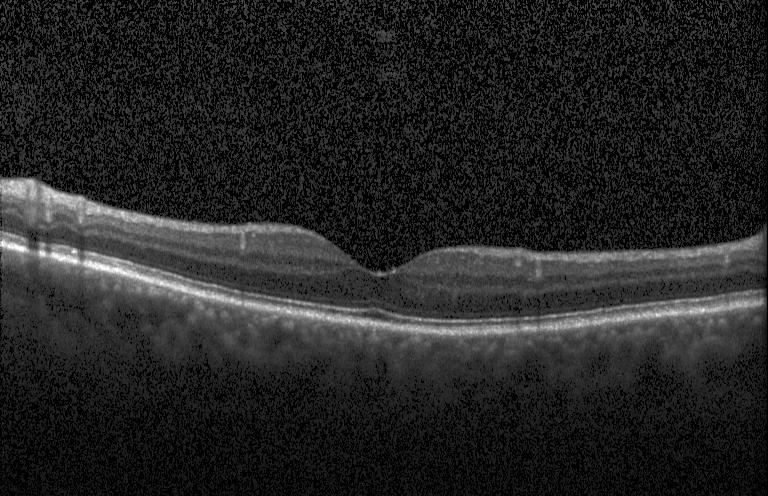

Spectral-domain OCT. Acquired on a Heidelberg Spectralis. OCT B-scan
OCT finding: no evidence of choroidal neovascularization, diabetic macular edema, or drusen.